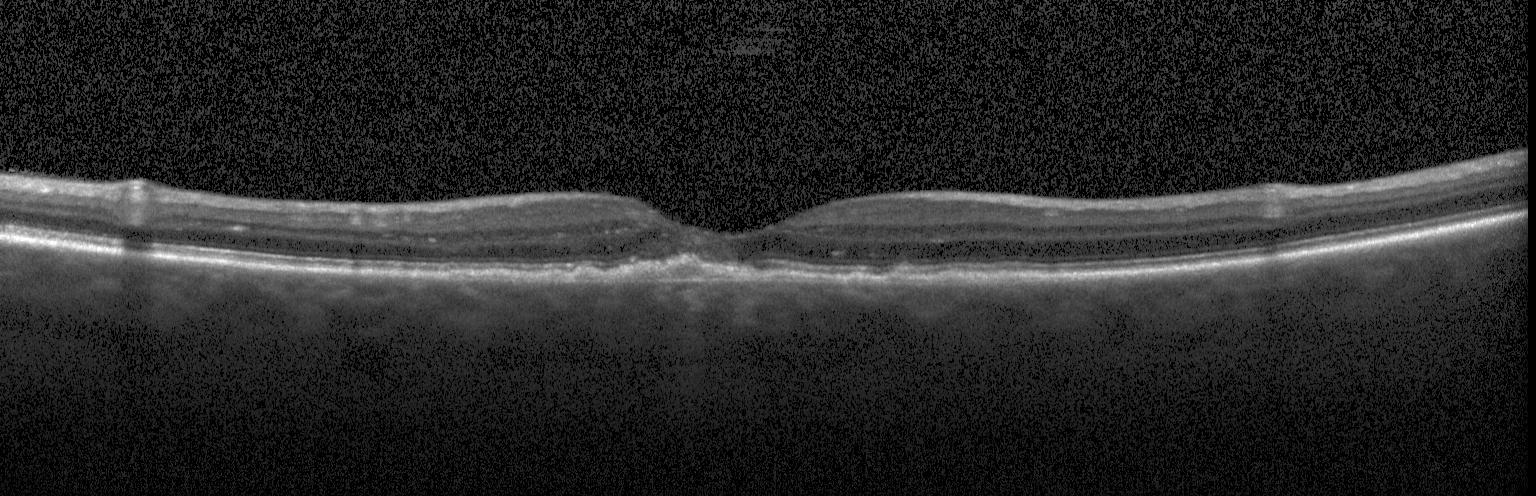 This B-scan demonstrates choroidal neovascularization.